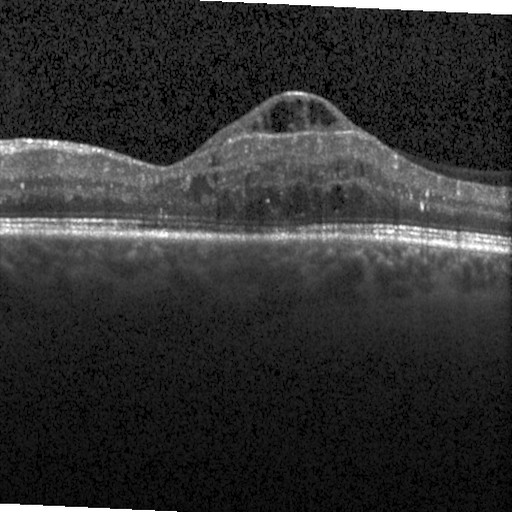
DME.